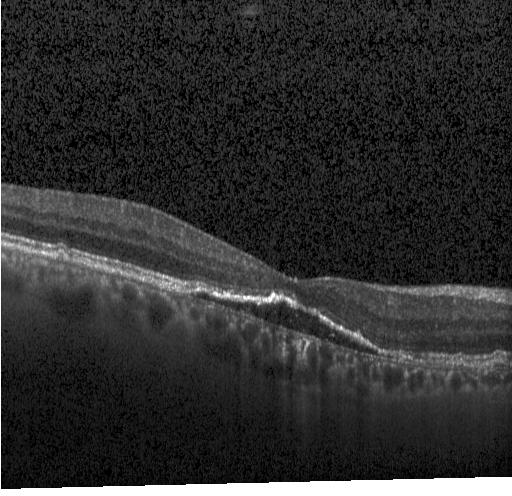
Spectral-domain OCT B-scan: a choroidal neovascular membrane.